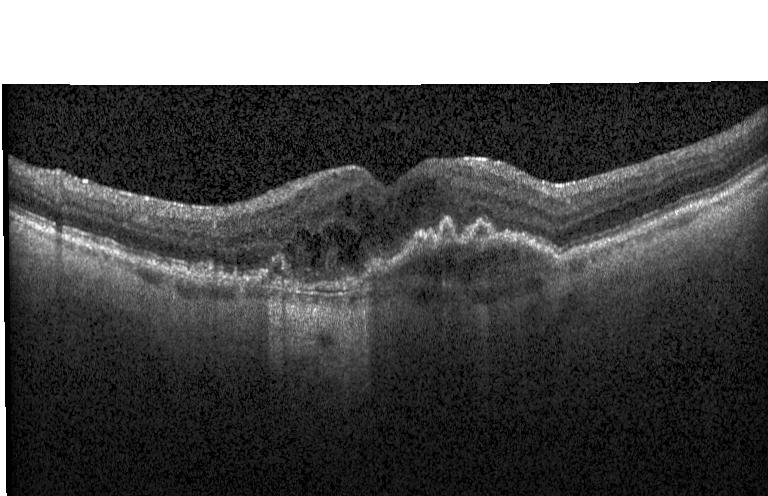

Through the macula · optical coherence tomography B-scan.
This B-scan demonstrates a choroidal neovascular membrane.